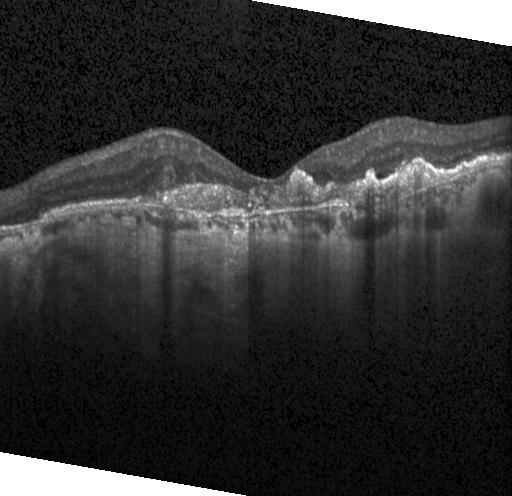

Retinal OCT cross-section
A choroidal neovascular membrane.